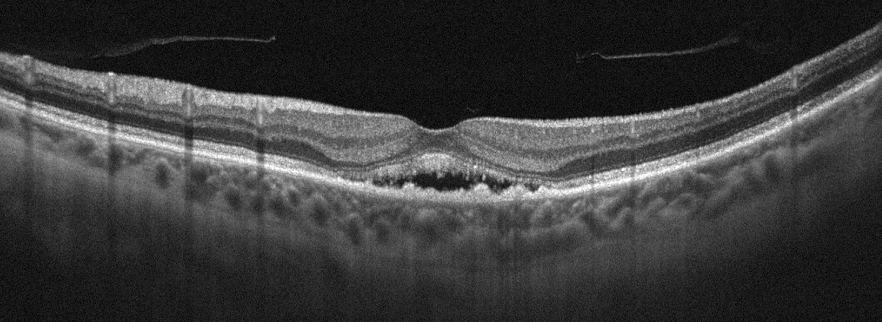

Macular OCT: age-related macular degeneration (AMD).